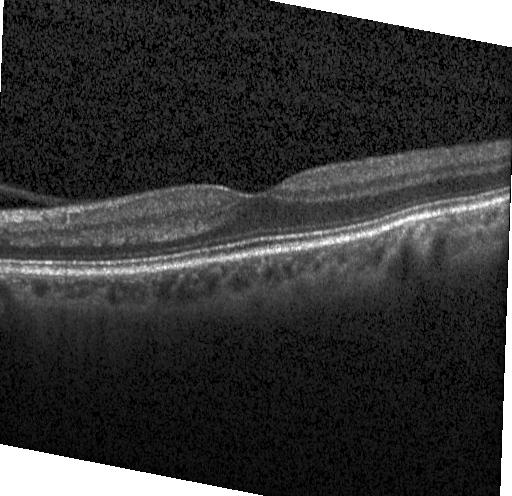

Centered on the fovea; spectral-domain optical coherence tomography; Heidelberg Spectralis OCT system; optical coherence tomography scan.
Finding: neither choroidal neovascularization, diabetic macular edema, nor drusen.